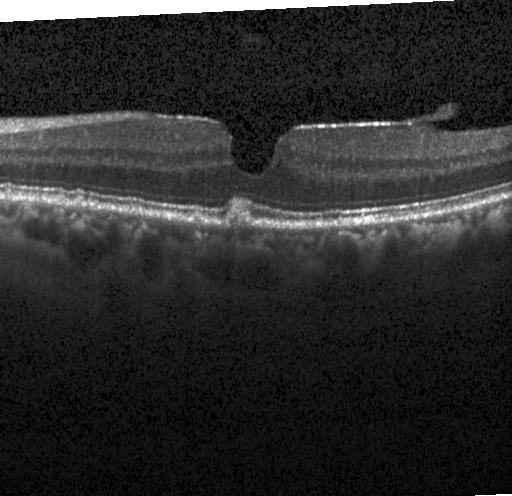

Finding: multiple drusen.